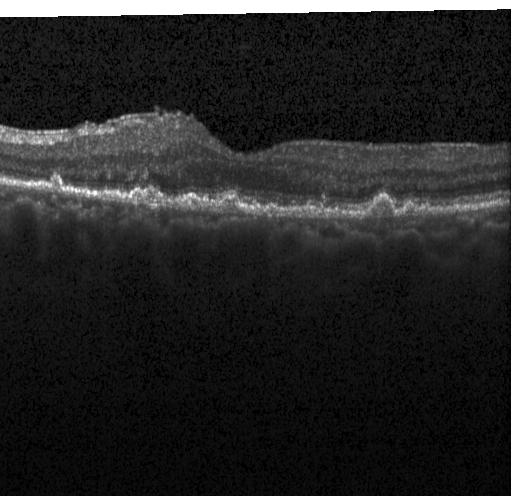
Retinal OCT cross-section, SD-OCT, through the macula, Heidelberg Spectralis OCT system. Diagnosis: sub-RPE drusenoid deposits.